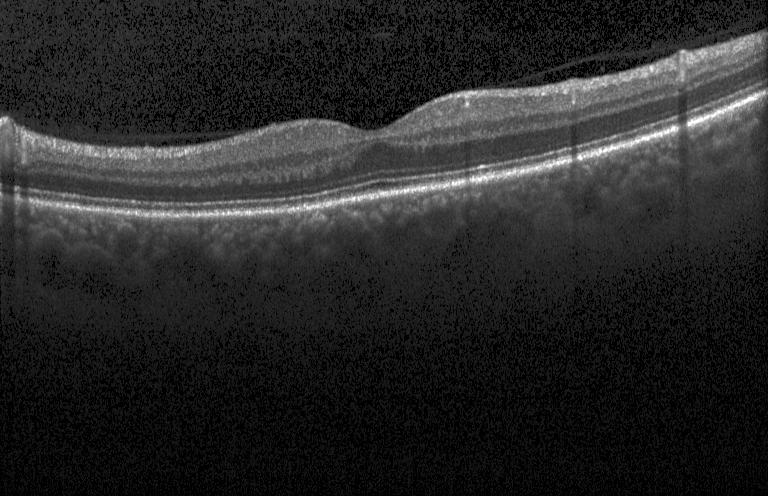 Optical coherence tomography scan — Macular OCT: neither choroidal neovascularization, diabetic macular edema, nor drusen.